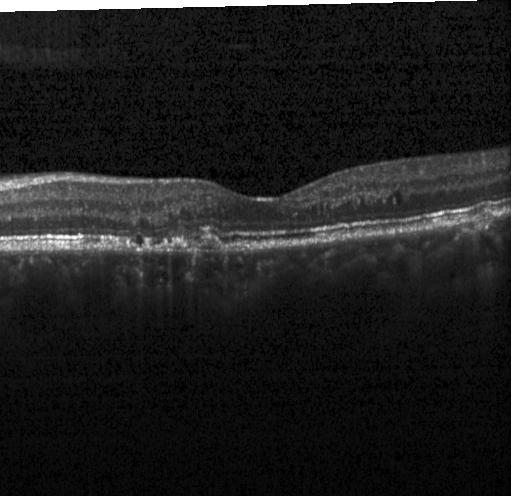

Centered on the fovea. Retinal OCT B-scan. Acquired on a Heidelberg Spectralis. Diagnosis: choroidal neovascularization (CNV).